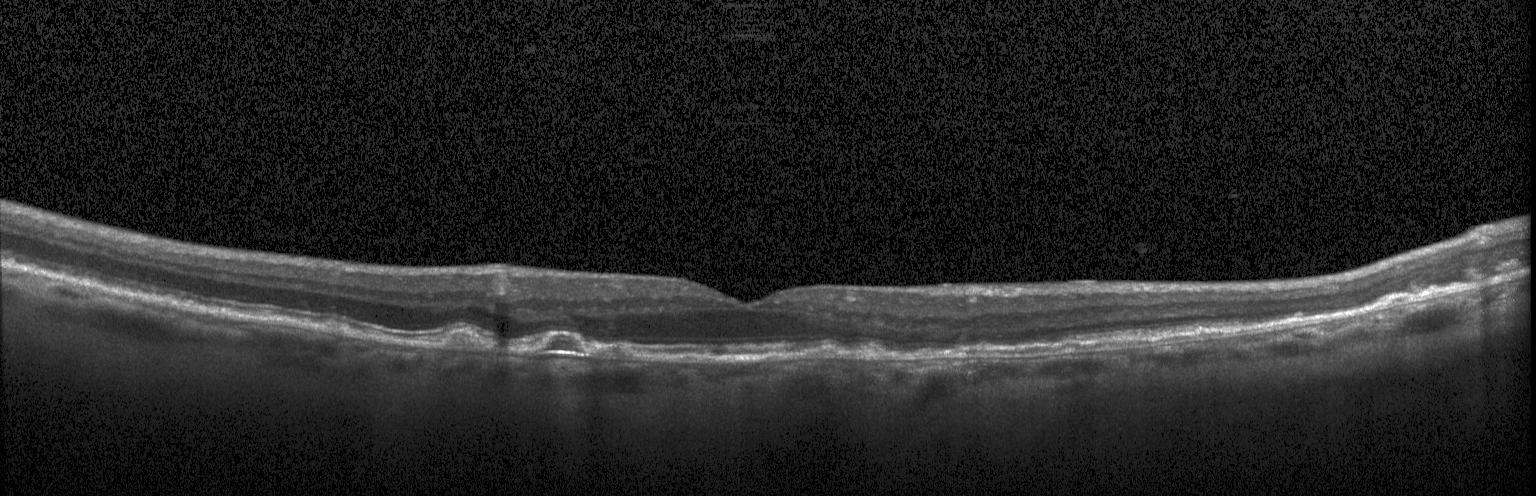

OCT B-scan. Horizontal scan through the fovea. Instrument: Heidelberg Spectralis
Impression: a choroidal neovascular membrane.